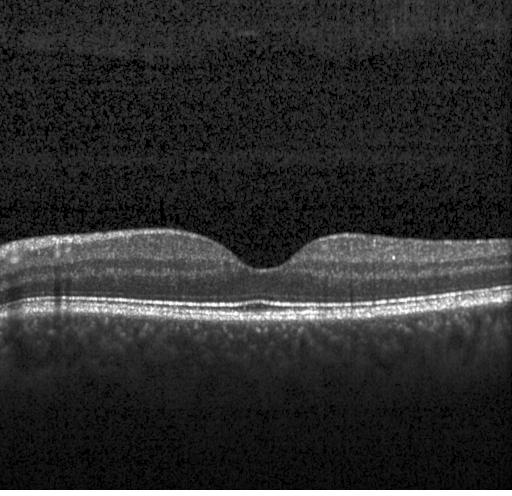
Retinal OCT cross-section showing no CNV, DME, or drusen.